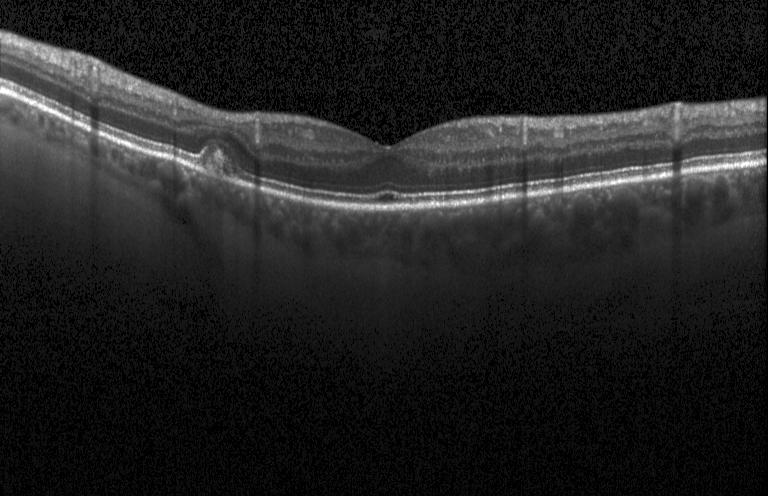

Finding: no evidence of CNV, DME, or drusen.